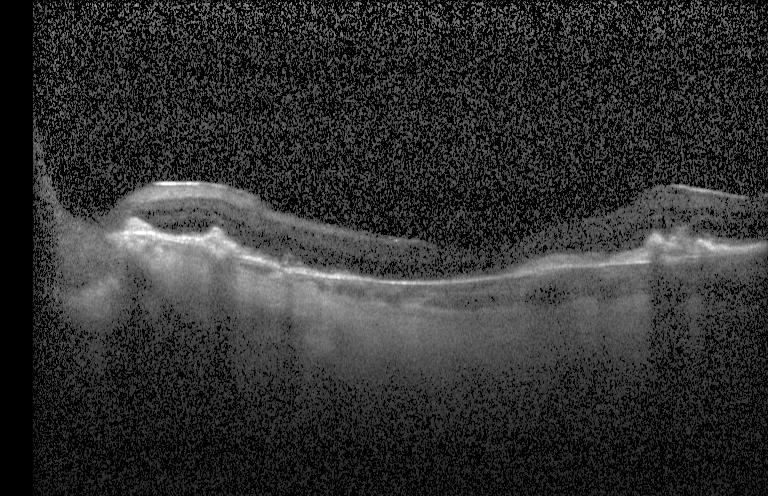

Acquired on a Heidelberg Spectralis, OCT line scan.
The scan shows a choroidal neovascular membrane.